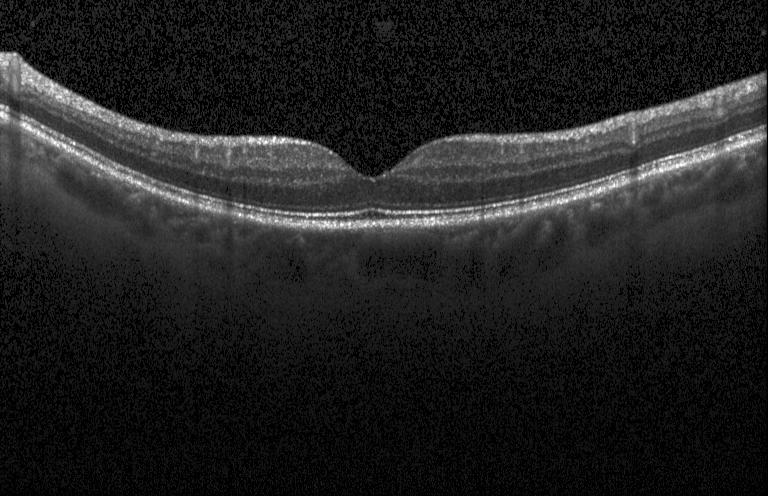 Heidelberg Spectralis. Spectral-domain optical coherence tomography. OCT B-scan
The scan shows no choroidal neovascularization, no diabetic macular edema, and no drusen.